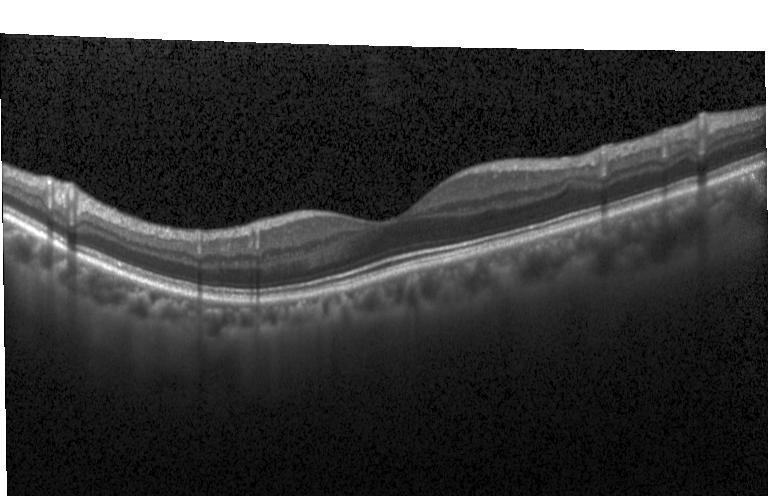
Impression: no choroidal neovascularization, no diabetic macular edema, and no drusen.